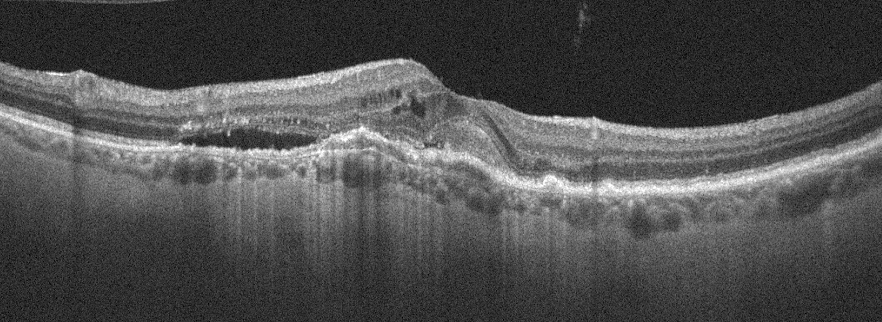

OS; optical coherence tomography scan. Diagnosis: age-related macular degeneration.